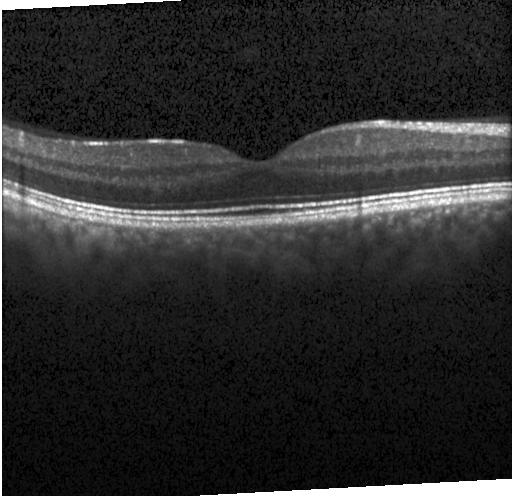 Horizontal scan through the fovea; spectral-domain OCT; Heidelberg Spectralis OCT system; retinal OCT cross-section.
Impression: no evidence of CNV, DME, or drusen.